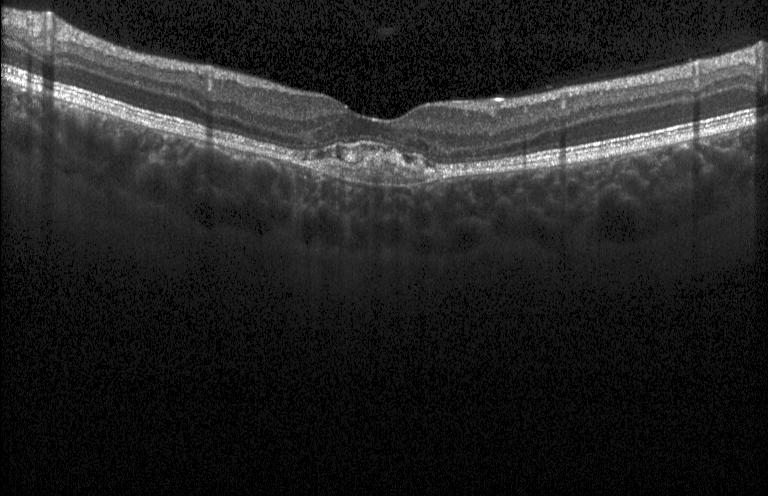 Finding: choroidal neovascularization (CNV).